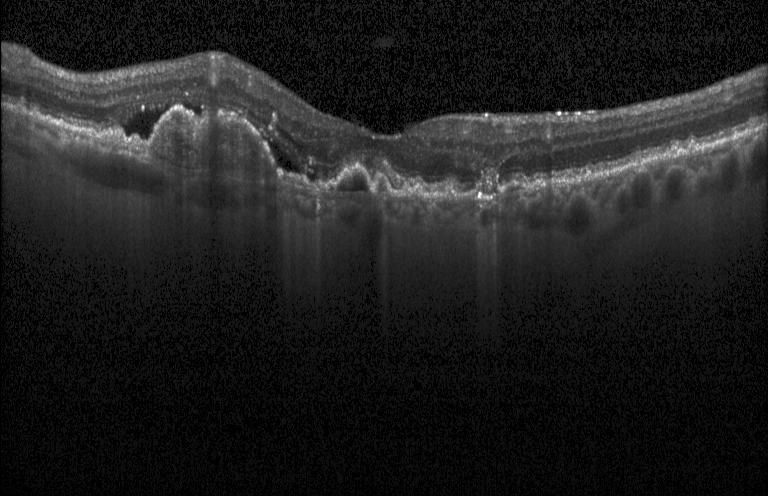 Retinal OCT B-scan; SD-OCT; instrument: Heidelberg Spectralis; fovea-centered
The scan shows CNV.